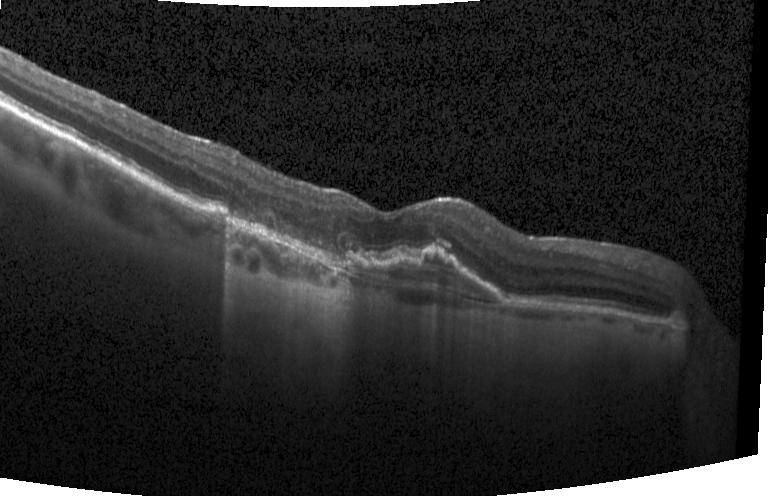
Diagnosis: a choroidal neovascular membrane.